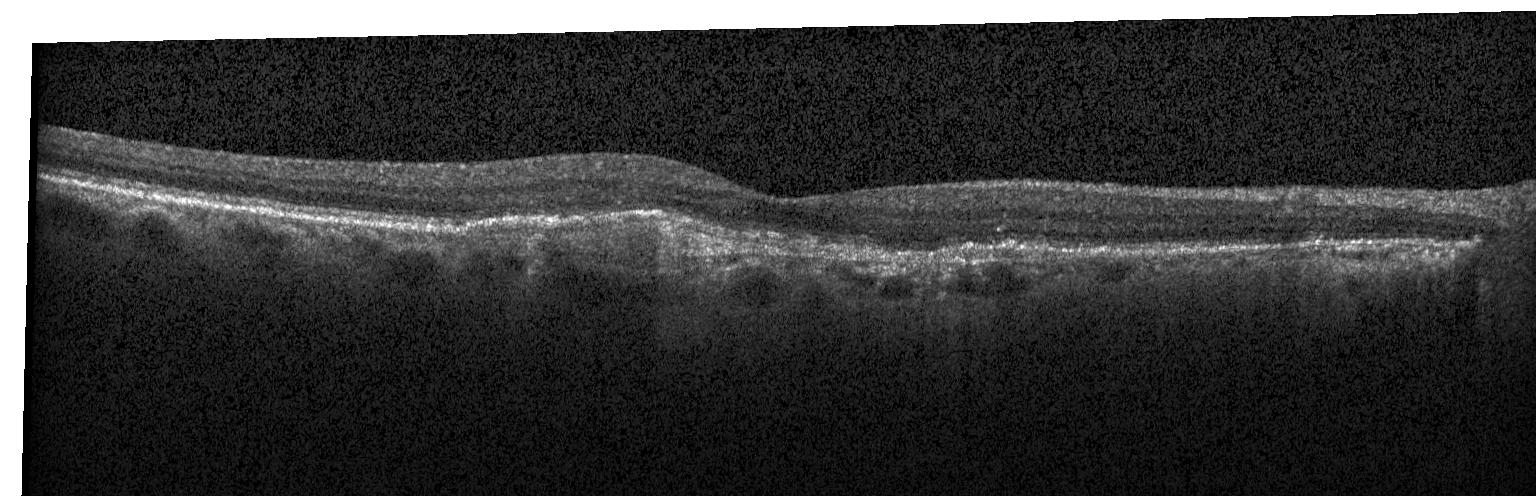 SD-OCT, OCT line scan.
Dx: a choroidal neovascular membrane.